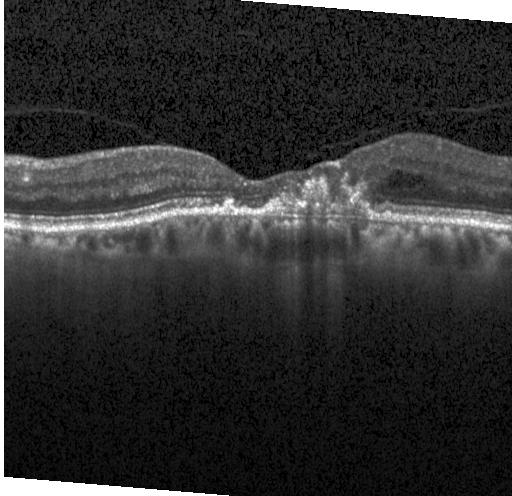
Impression: choroidal neovascularization.